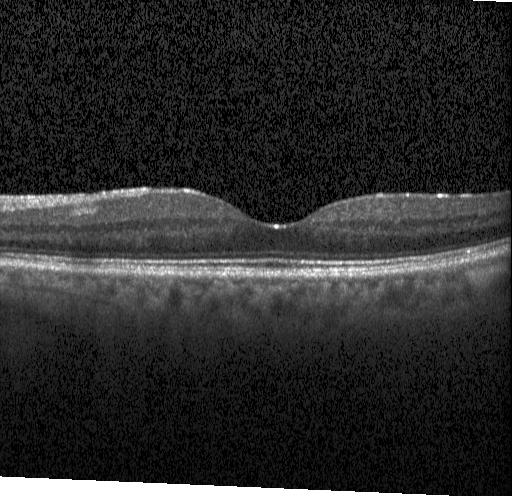
Spectral-domain OCT · instrument: Heidelberg Spectralis · optical coherence tomography B-scan — Finding: no choroidal neovascularization, no diabetic macular edema, and no drusen.